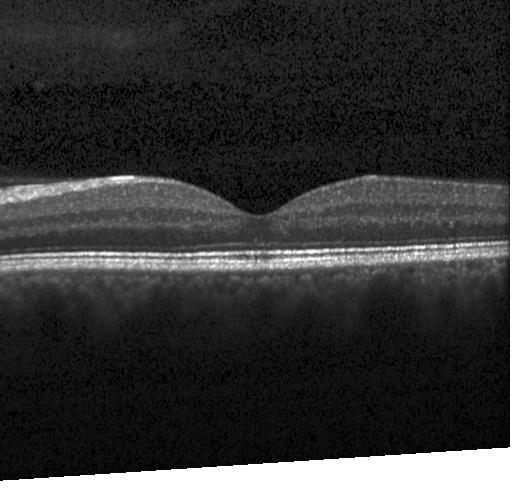
Retinal OCT cross-section showing no CNV, DME, or drusen.